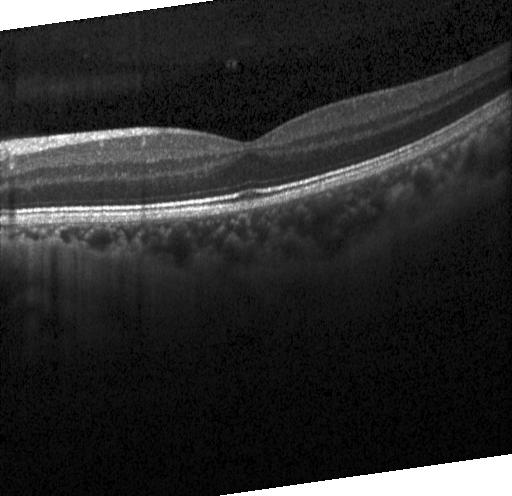

Finding: no choroidal neovascularization, no diabetic macular edema, and no drusen.